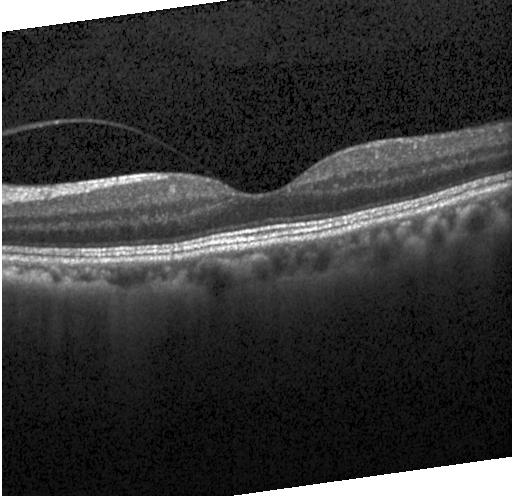

Dx: neither CNV, DME, nor drusen.